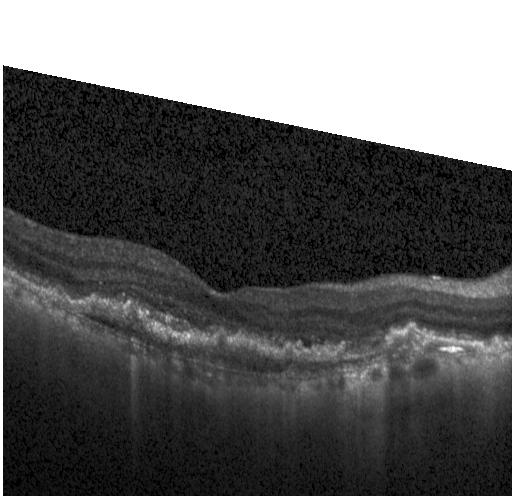

Retinal OCT cross-section
Finding: choroidal neovascularization (CNV).